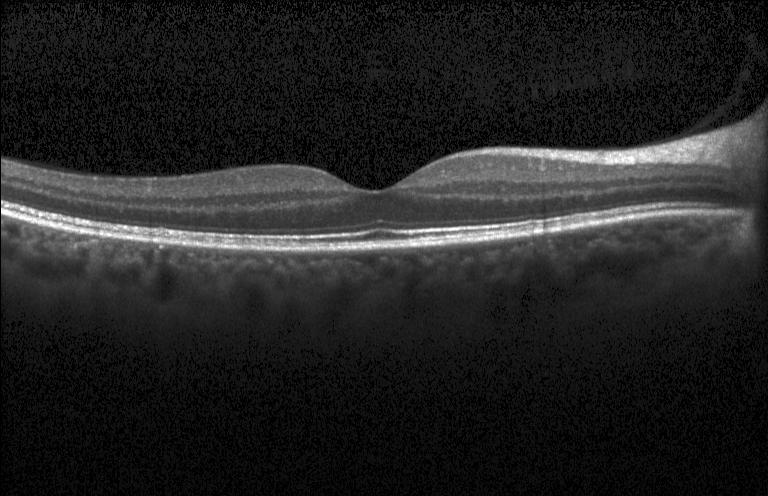
Spectral-domain optical coherence tomography, centered on the fovea, retinal OCT B-scan.
The scan shows no choroidal neovascularization, diabetic macular edema, or drusen.